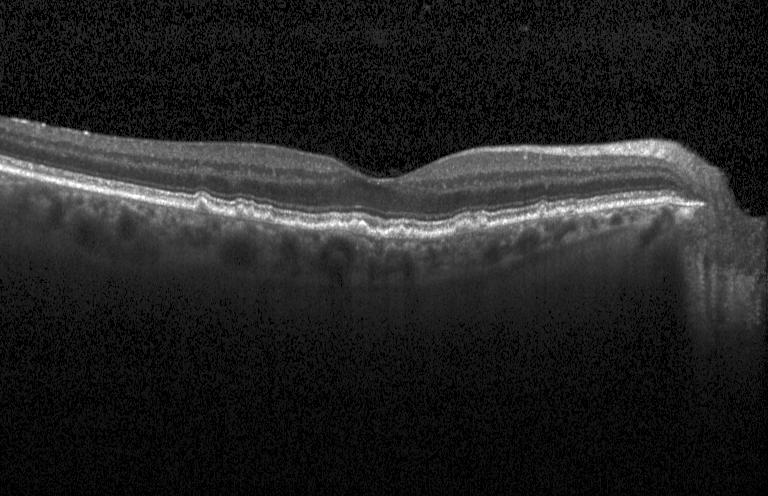 OCT line scan; centered on the fovea; instrument: Heidelberg Spectralis; SD-OCT. The scan shows sub-RPE drusenoid deposits.